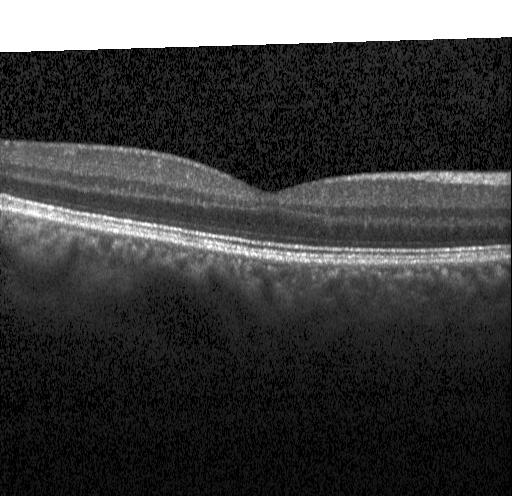
Impression: neither choroidal neovascularization, diabetic macular edema, nor drusen.